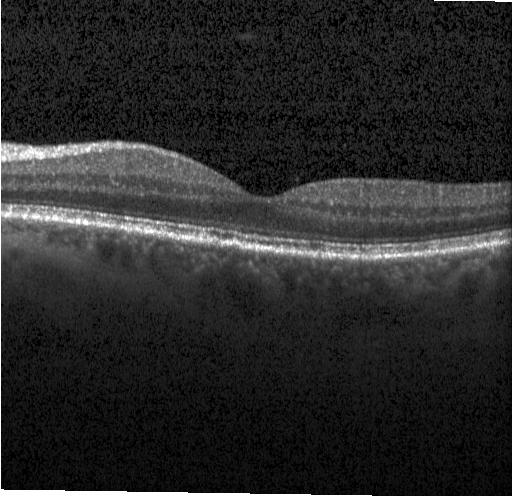 This B-scan demonstrates no choroidal neovascularization, diabetic macular edema, or drusen.